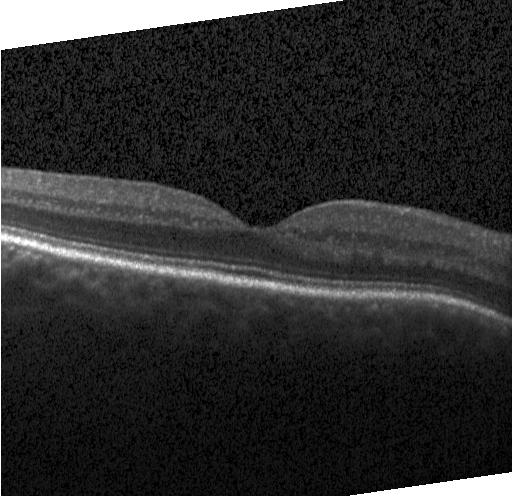

OCT B-scan · SD-OCT — OCT finding: no evidence of CNV, DME, or drusen.